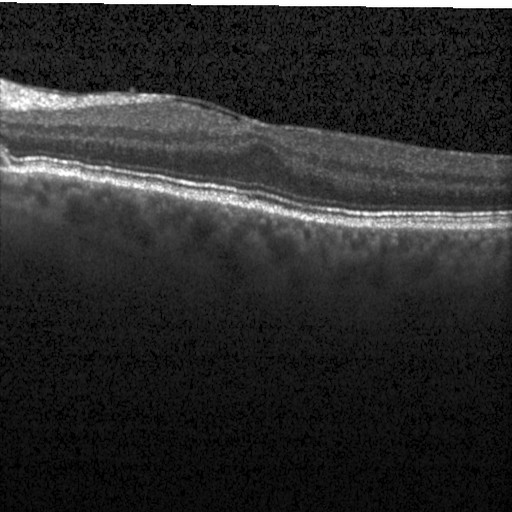 OCT B-scan, Heidelberg Spectralis OCT system, SD-OCT.
Assessment: diabetic macular edema (DME).